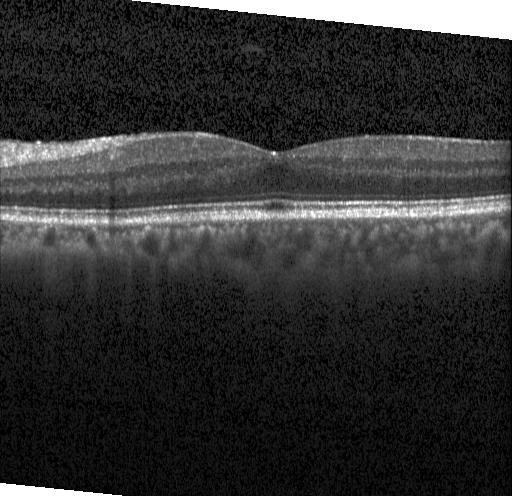 Retinal OCT cross-section showing no choroidal neovascularization, diabetic macular edema, or drusen.